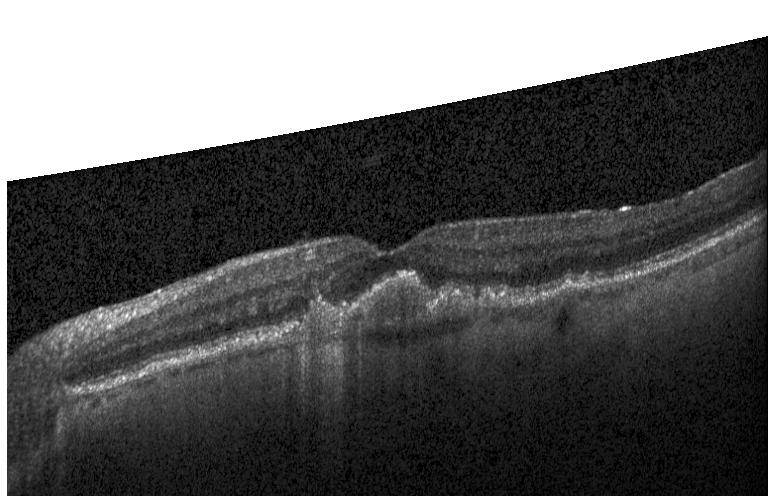 Through the macula · optical coherence tomography B-scan · spectral-domain optical coherence tomography · Heidelberg Spectralis OCT system. Dx: CNV.